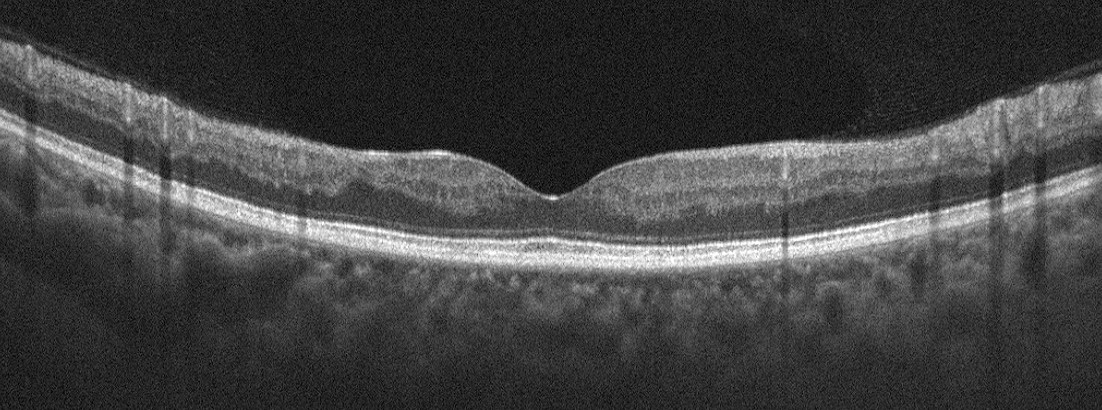
Macular scan · optical coherence tomography B-scan.
Dx: retinal vein occlusion.